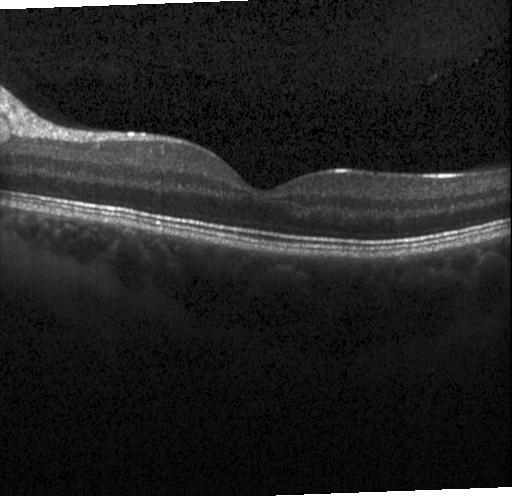

Finding: no CNV, no DME, and no drusen.